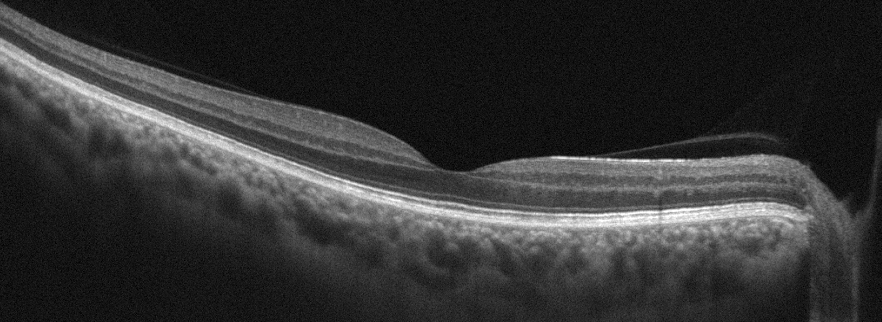
Through the macula; optical coherence tomography B-scan; oculus dexter; instrument: Optovue Avanti RTVue XR. OCT finding: no AMD, DME, ERM, RAO, RVO, or VID.